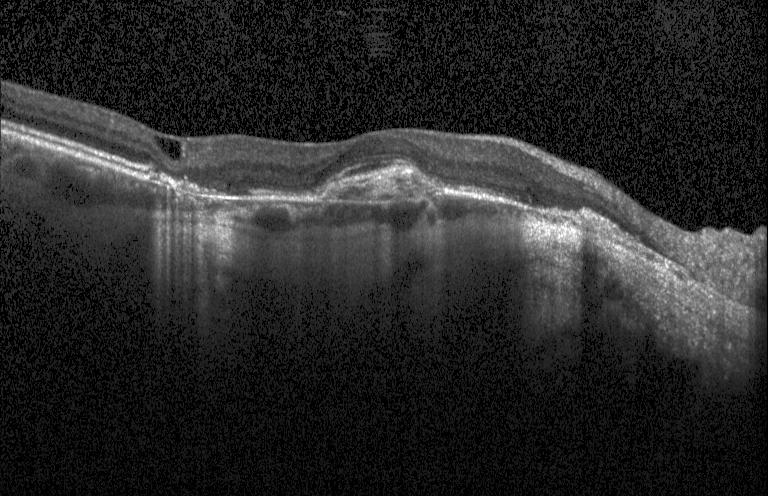

Spectral-domain OCT, retinal OCT B-scan, Heidelberg Spectralis, macular scan — Diagnosis: CNV.